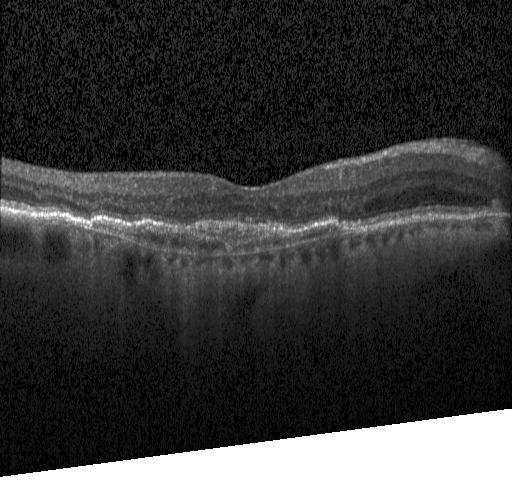
Optical coherence tomography scan.
Diagnosis: a choroidal neovascular membrane.